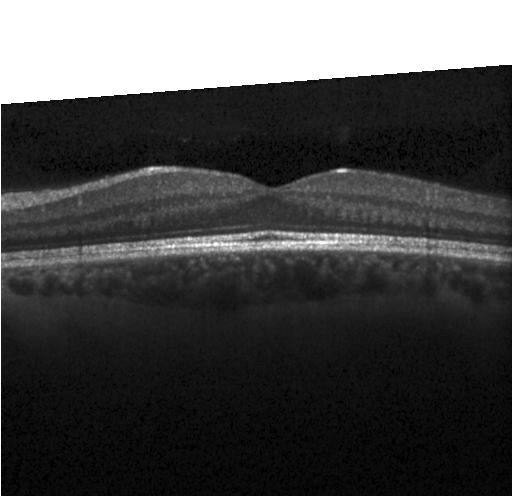
Optical coherence tomography scan
OCT finding: no choroidal neovascularization, diabetic macular edema, or drusen.